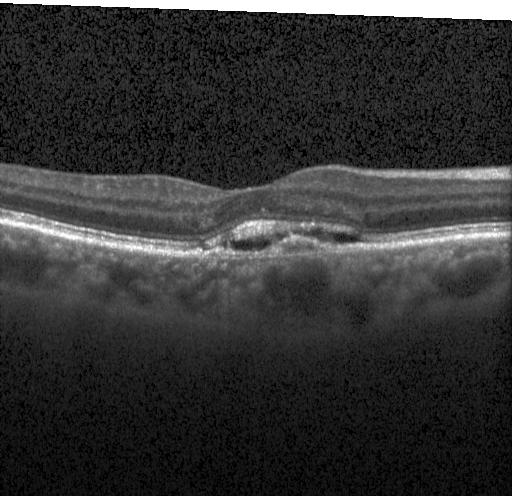
Retinal OCT cross-section showing a choroidal neovascular membrane.